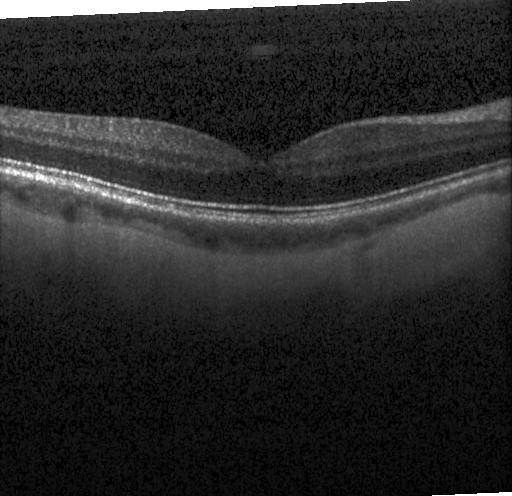

Spectral-domain OCT B-scan: no evidence of CNV, DME, or drusen.